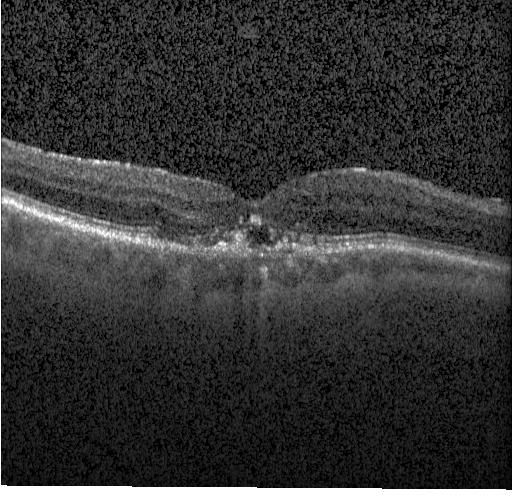
Horizontal scan through the fovea · OCT B-scan
Diagnosis: choroidal neovascularization (CNV).